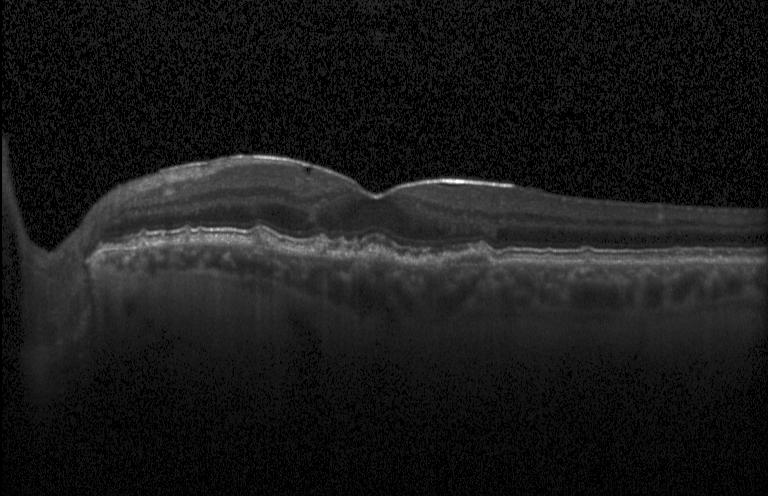 Optical coherence tomography B-scan · SD-OCT · macular scan
The scan shows sub-RPE drusenoid deposits.